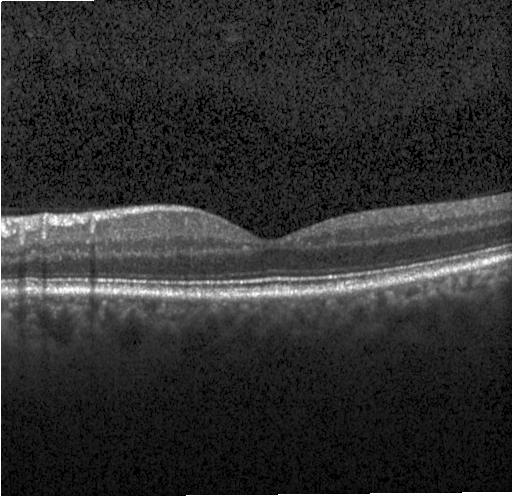 Retinal OCT cross-section showing no CNV, DME, or drusen.